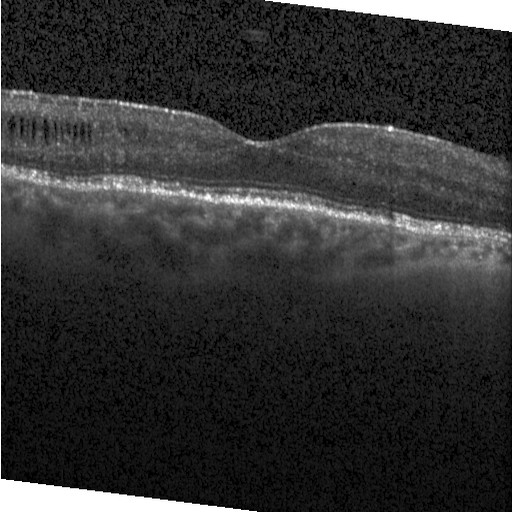

Macular OCT demonstrating diabetic macular edema (DME).